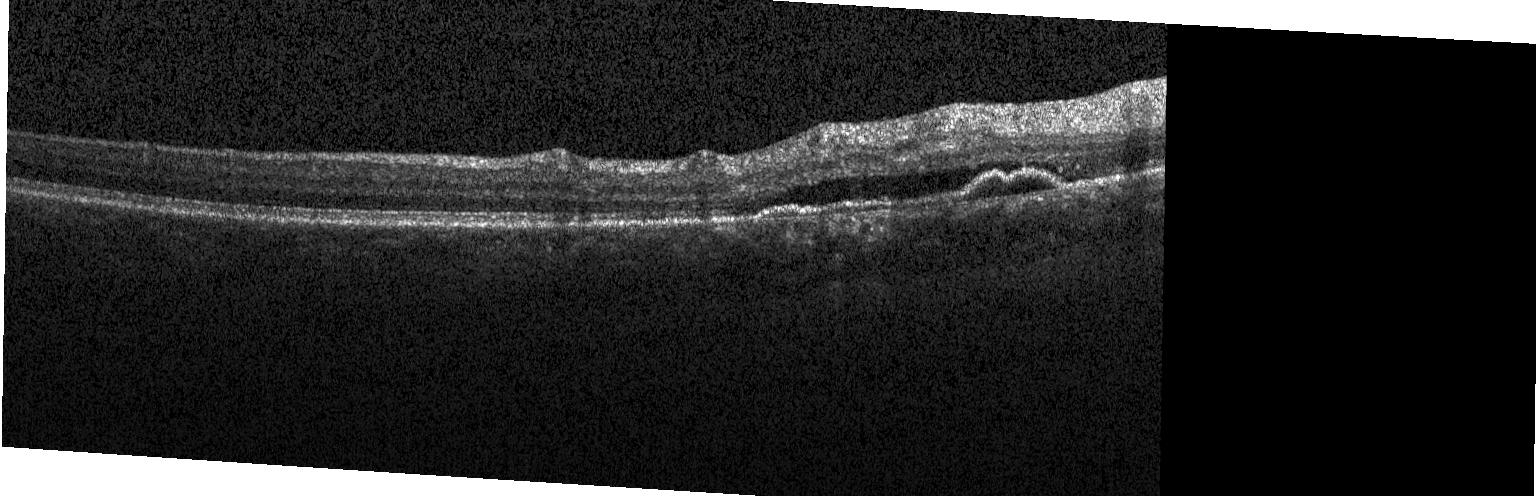 Spectral-domain OCT B-scan: choroidal neovascularization.